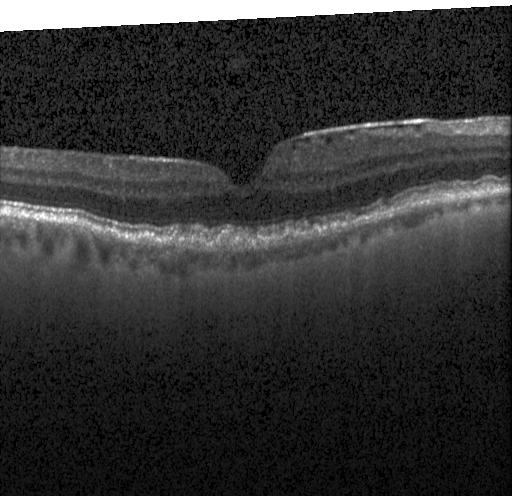 Horizontal scan through the fovea; optical coherence tomography B-scan — This B-scan demonstrates multiple drusen.